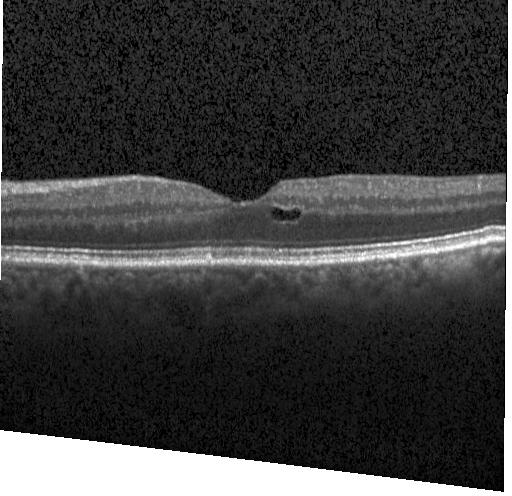 Diagnosis: diabetic macular edema (DME).